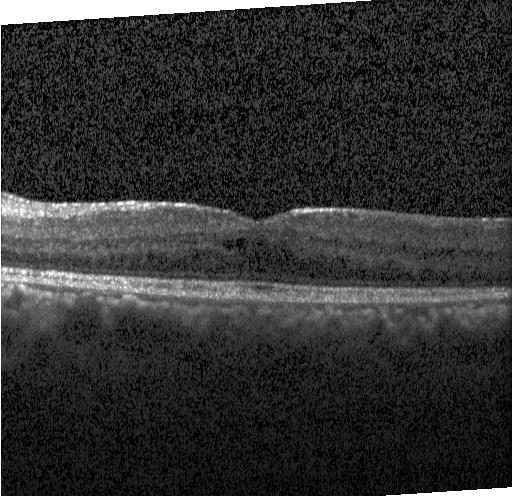

Horizontal scan through the fovea · retinal OCT B-scan · spectral-domain OCT. Impression: diabetic macular edema.